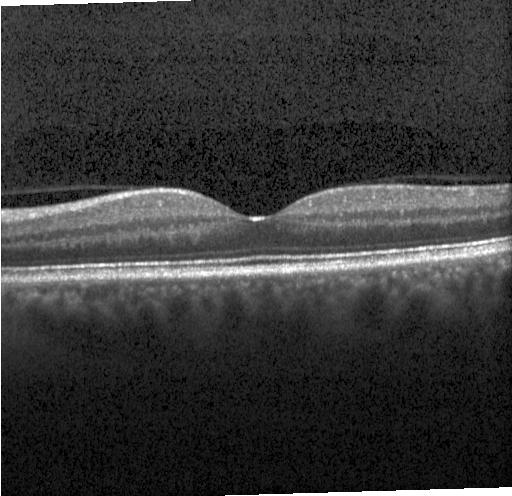 OCT B-scan showing no choroidal neovascularization, diabetic macular edema, or drusen.